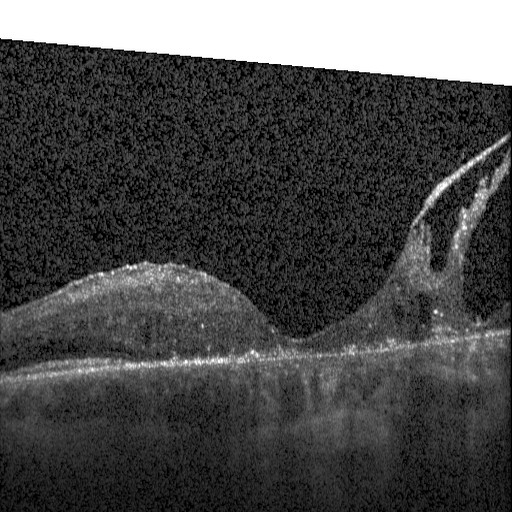 Diagnosis: DME.